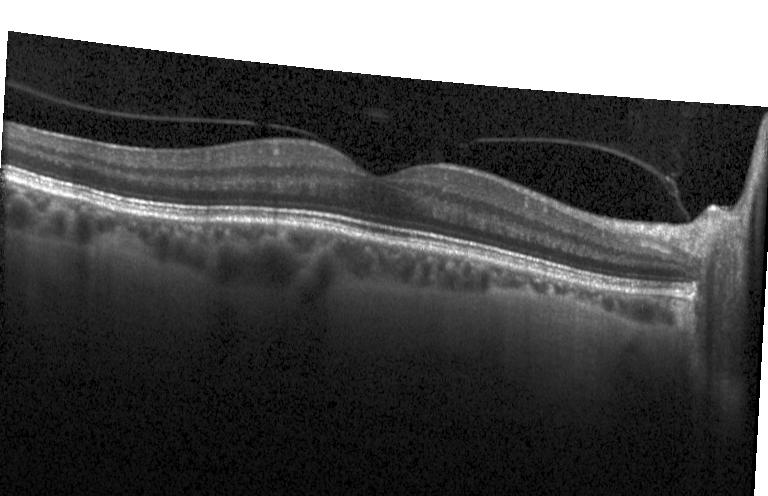

No choroidal neovascularization, no diabetic macular edema, and no drusen.